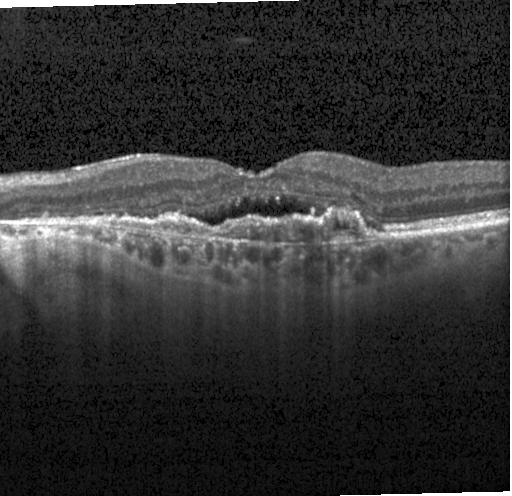

OCT B-scan — This B-scan demonstrates CNV.